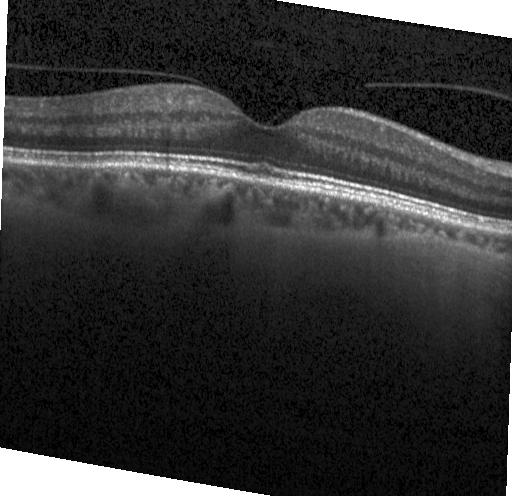

Finding: neither CNV, DME, nor drusen.